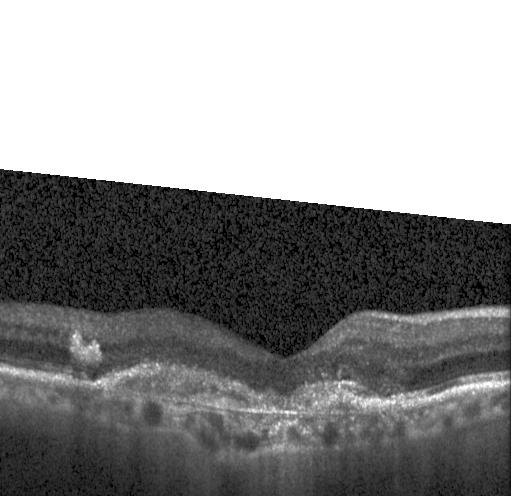
OCT line scan; fovea-centered; spectral-domain optical coherence tomography; instrument: Heidelberg Spectralis — This B-scan demonstrates choroidal neovascularization.